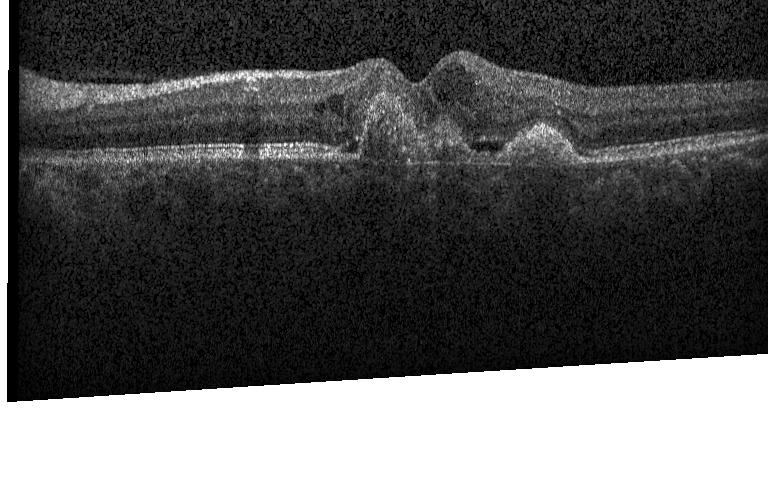

Retinal OCT cross-section. OCT finding: choroidal neovascularization (CNV).